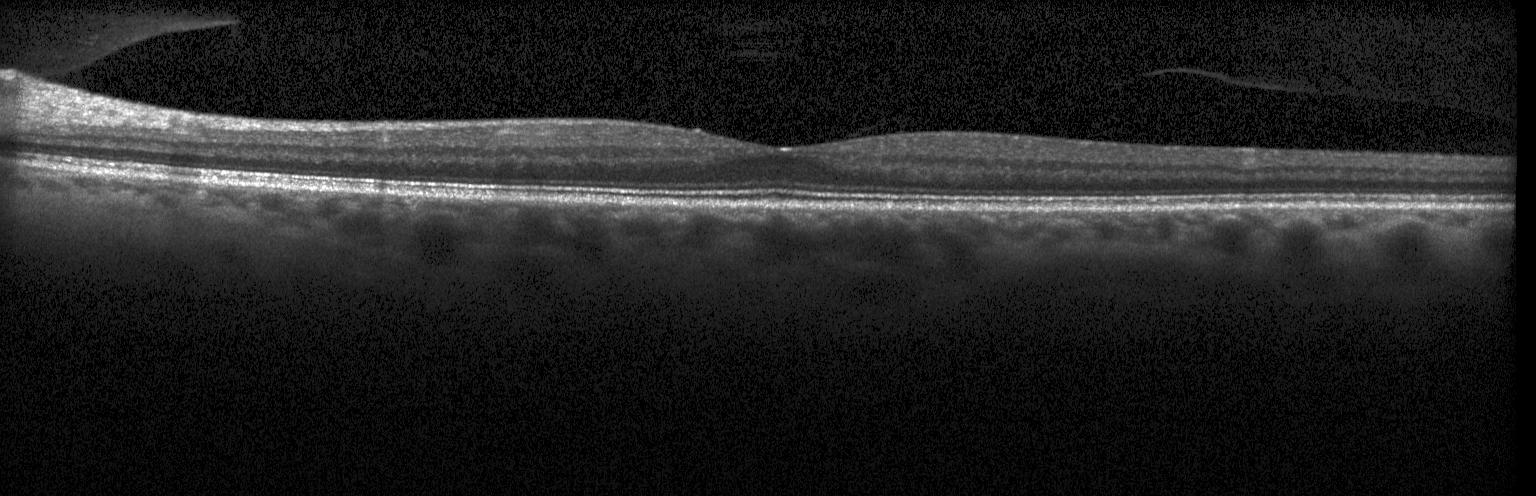 OCT finding: no choroidal neovascularization, no diabetic macular edema, and no drusen.